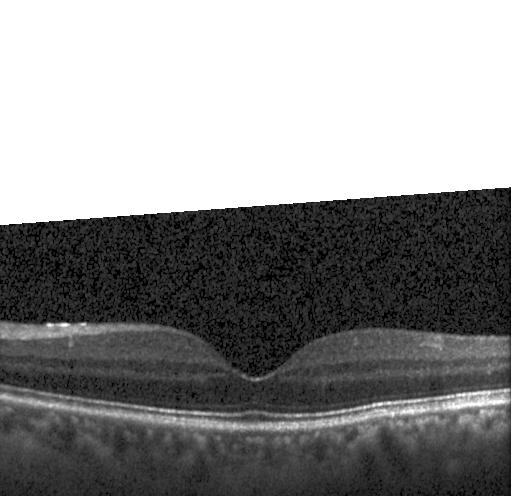 Retinal OCT B-scan; Heidelberg Spectralis; centered on the fovea; spectral-domain optical coherence tomography.
Impression: no evidence of choroidal neovascularization, diabetic macular edema, or drusen.